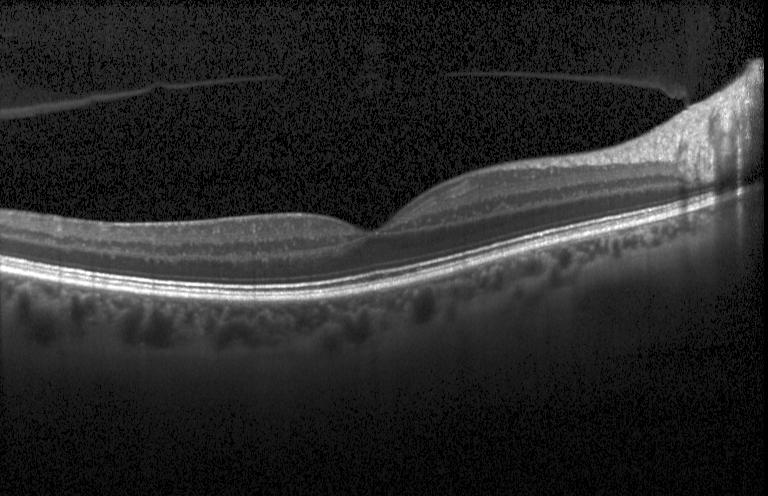 Fovea-centered, retinal OCT cross-section
Diagnosis: no CNV, no DME, and no drusen.